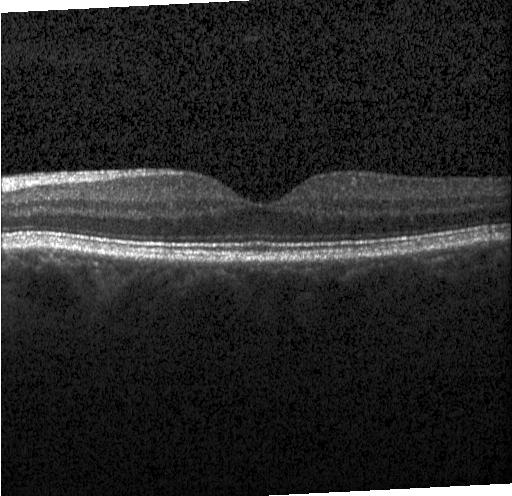

OCT line scan, centered on the fovea.
No CNV, no DME, and no drusen.